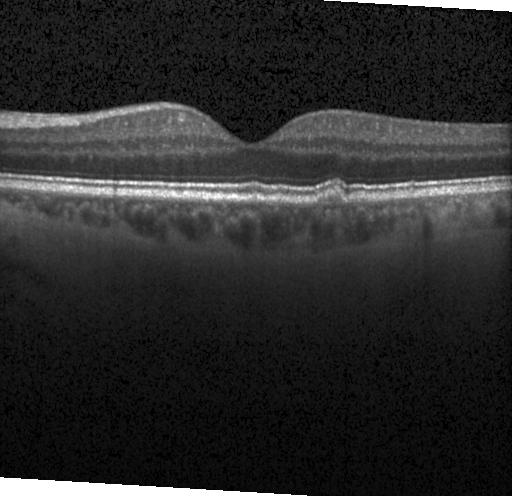
Retinal OCT cross-section · fovea-centered
The scan shows drusen.